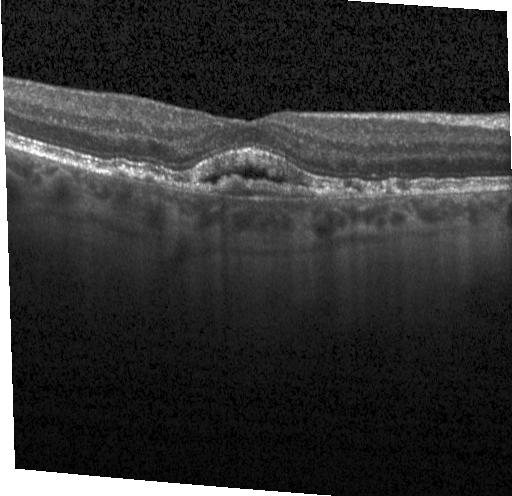
Macular scan · Heidelberg Spectralis · retinal OCT B-scan · spectral-domain optical coherence tomography
Finding: a choroidal neovascular membrane.